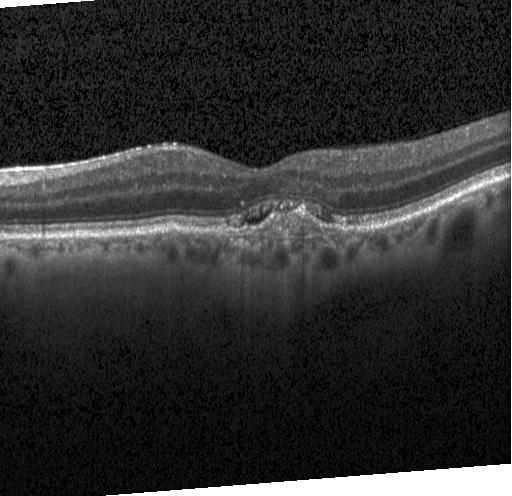
Retinal OCT B-scan · horizontal scan through the fovea.
A choroidal neovascular membrane.